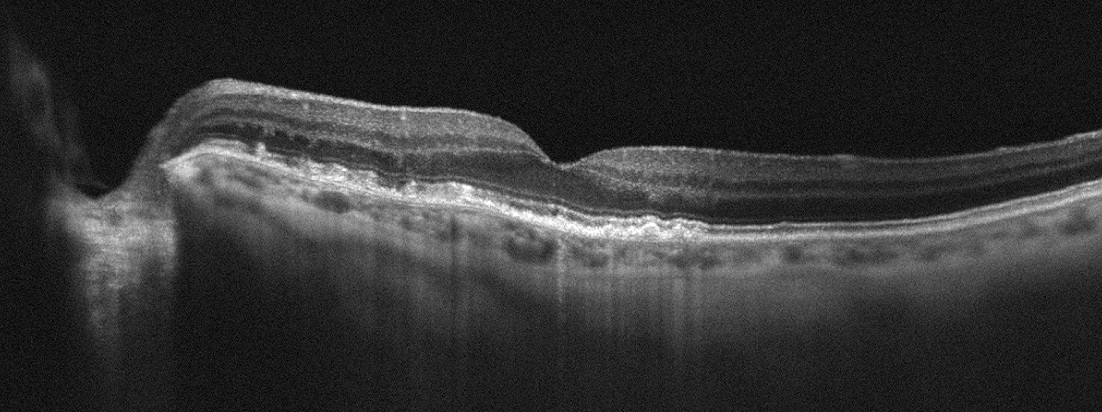
Diagnosis: AMD.